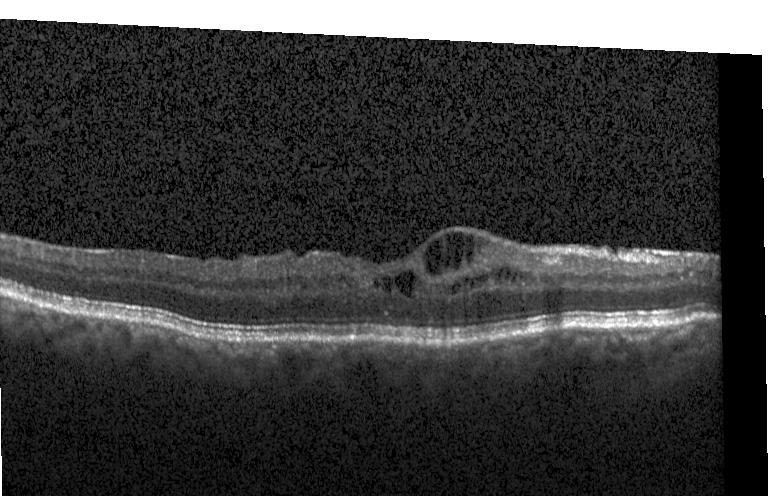

Diagnosis: diabetic macular edema.